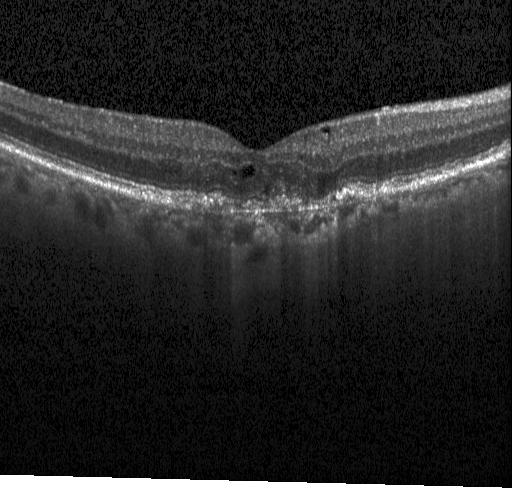

OCT B-scan · acquired on a Heidelberg Spectralis · centered on the fovea. OCT finding: CNV.